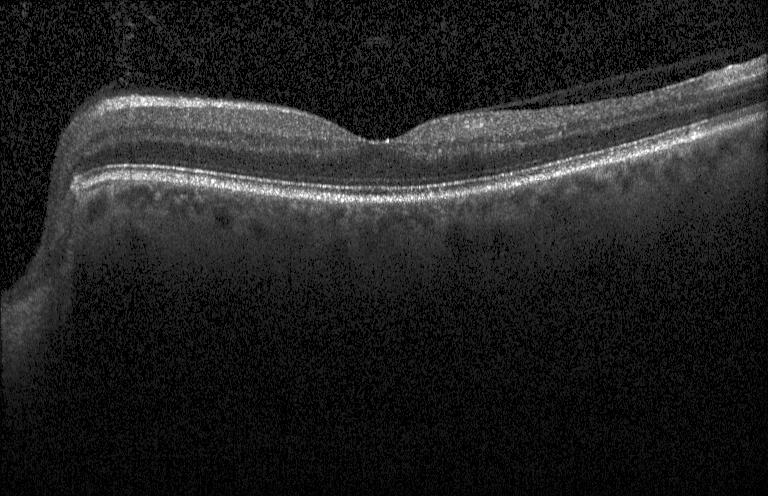
Finding: no evidence of choroidal neovascularization, diabetic macular edema, or drusen.